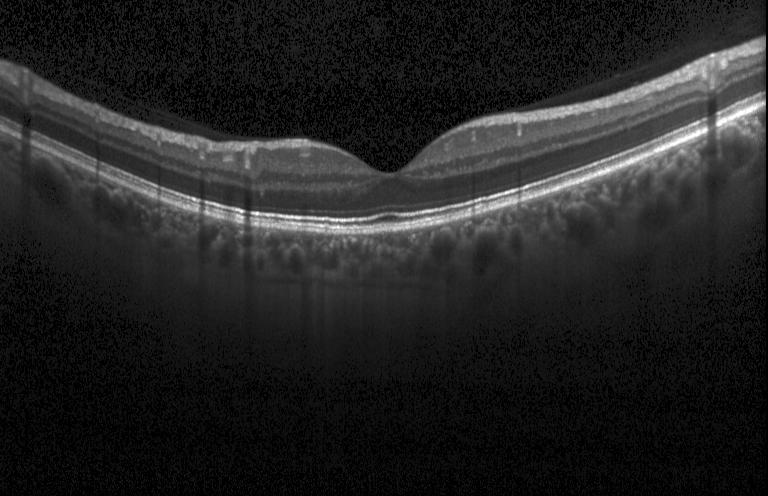

OCT finding: no choroidal neovascularization, diabetic macular edema, or drusen.